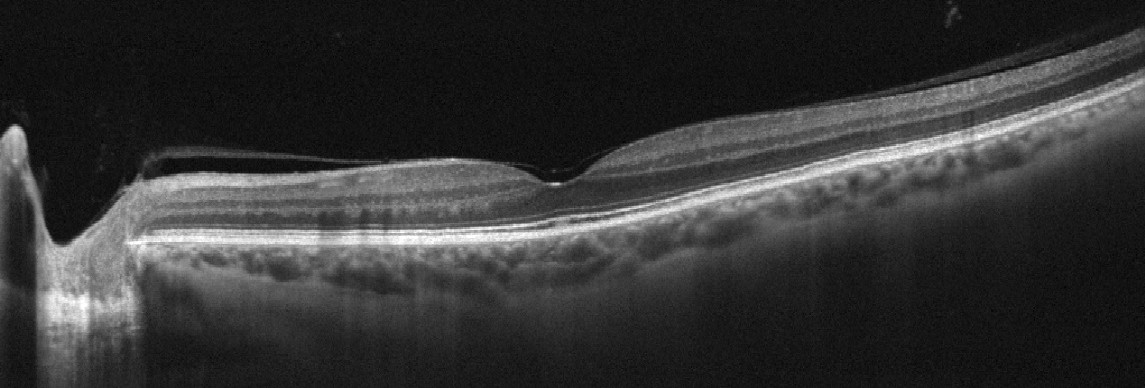
Finding: absence of AMD, DME, ERM, RAO, RVO, and vitreomacular interface disease.